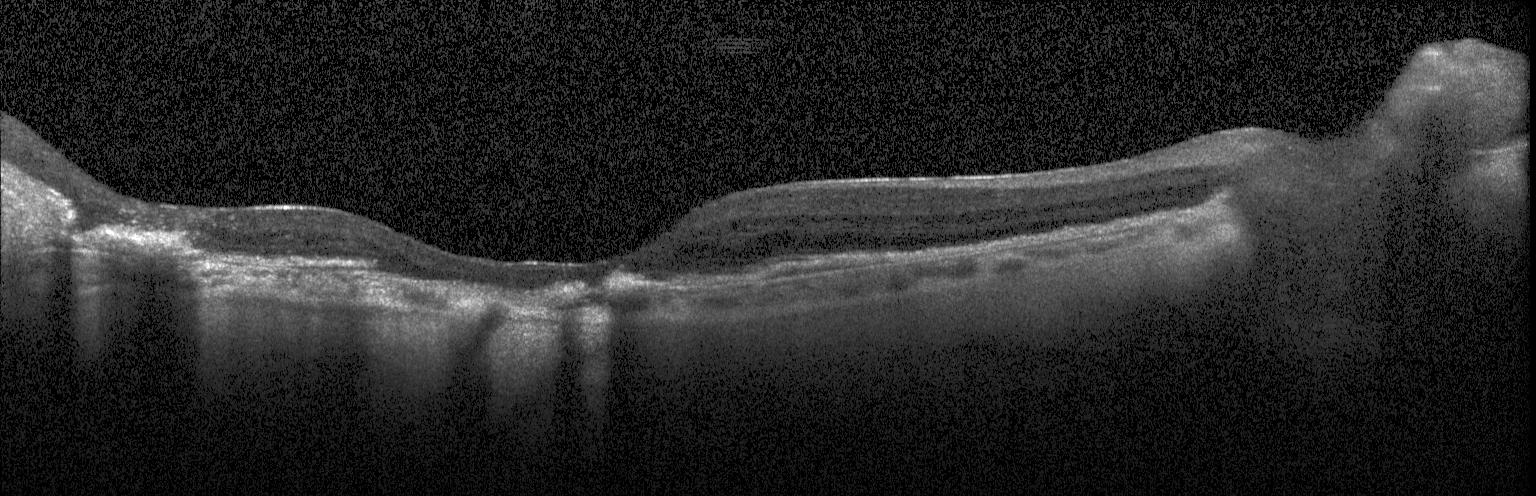 Centered on the fovea; OCT line scan
Finding: a choroidal neovascular membrane.